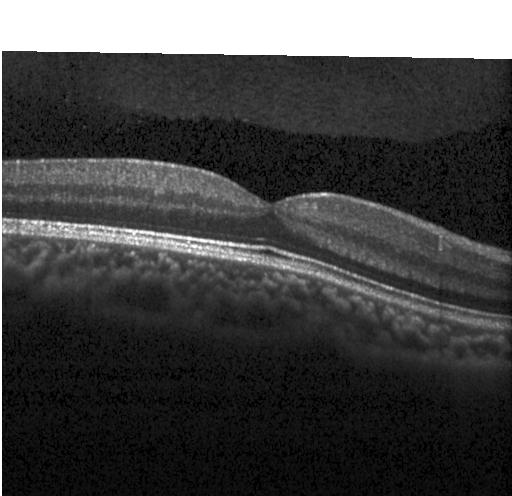

OCT finding: neither CNV, DME, nor drusen.